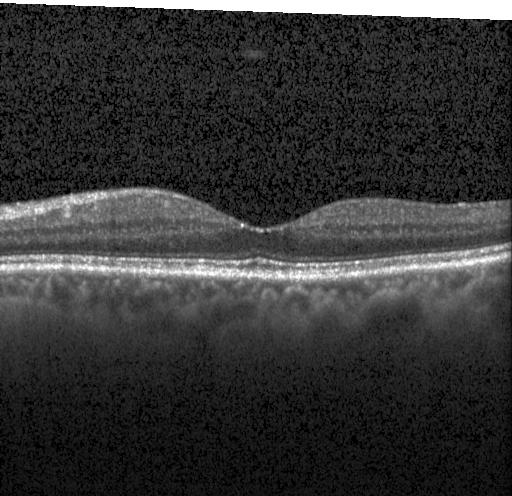 Dx: neither choroidal neovascularization, diabetic macular edema, nor drusen.